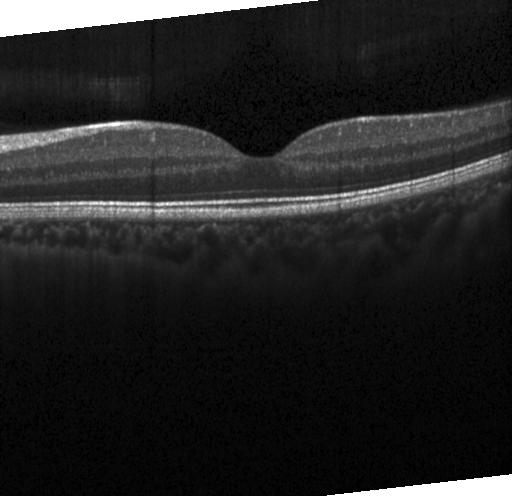
Optical coherence tomography B-scan, SD-OCT. This B-scan demonstrates no evidence of choroidal neovascularization, diabetic macular edema, or drusen.